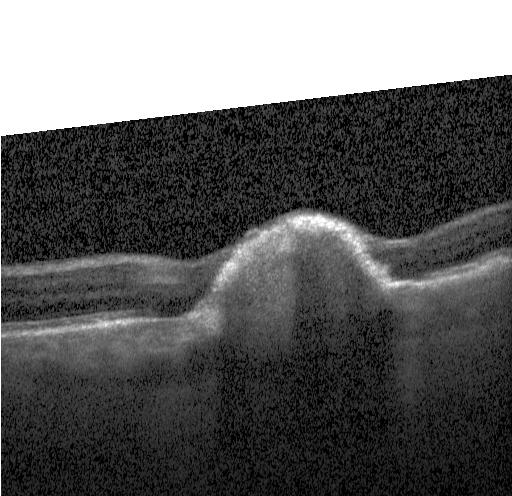
Finding: choroidal neovascularization.